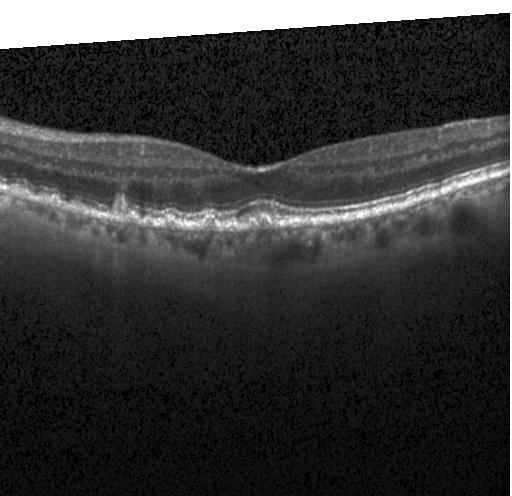

Heidelberg Spectralis, retinal OCT B-scan, macular scan — Multiple drusen.